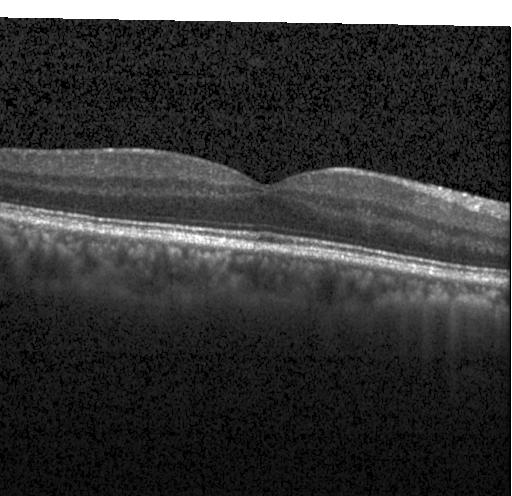

OCT scan showing neither choroidal neovascularization, diabetic macular edema, nor drusen.